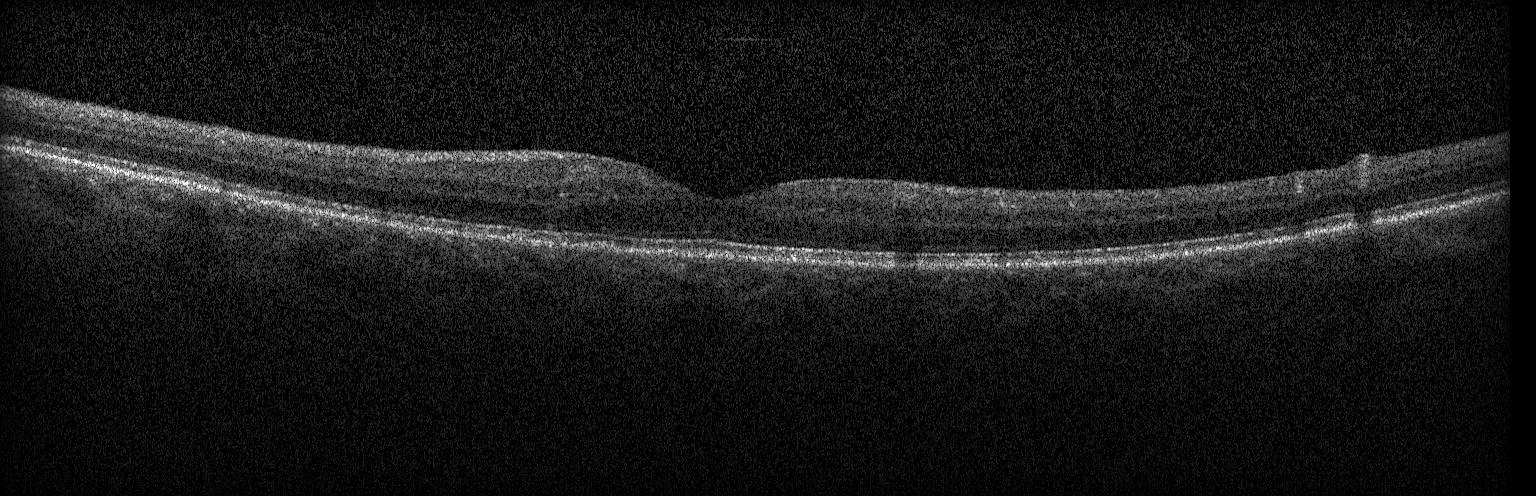 Impression: no evidence of choroidal neovascularization, diabetic macular edema, or drusen.